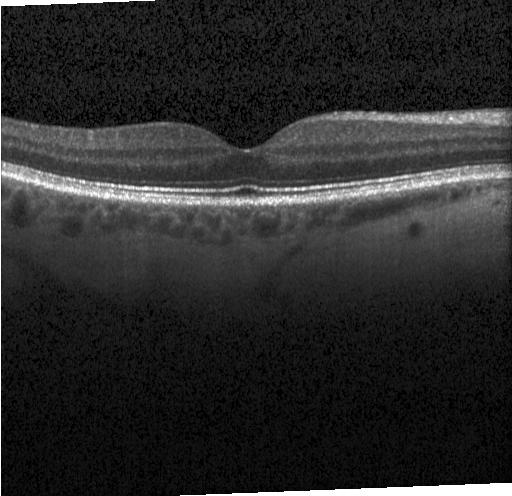
OCT scan showing no choroidal neovascularization, diabetic macular edema, or drusen.